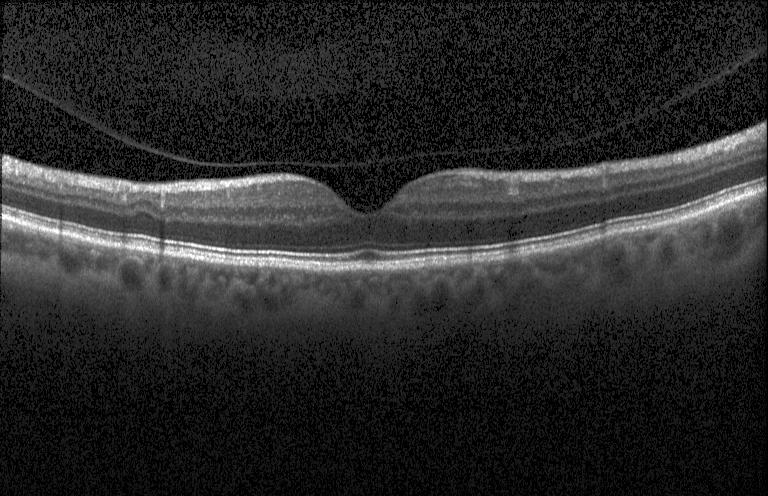
Dx: no CNV, no DME, and no drusen.